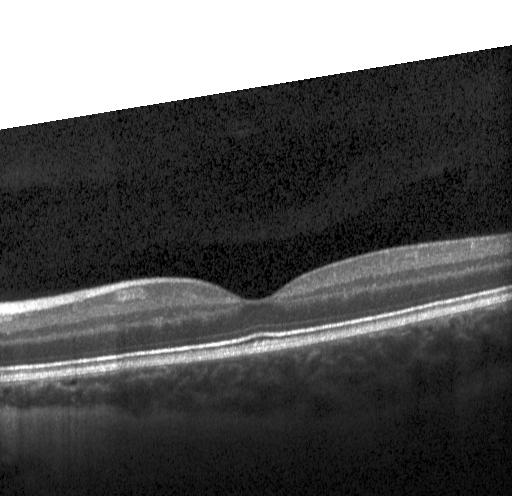 Dx: no evidence of choroidal neovascularization, diabetic macular edema, or drusen.